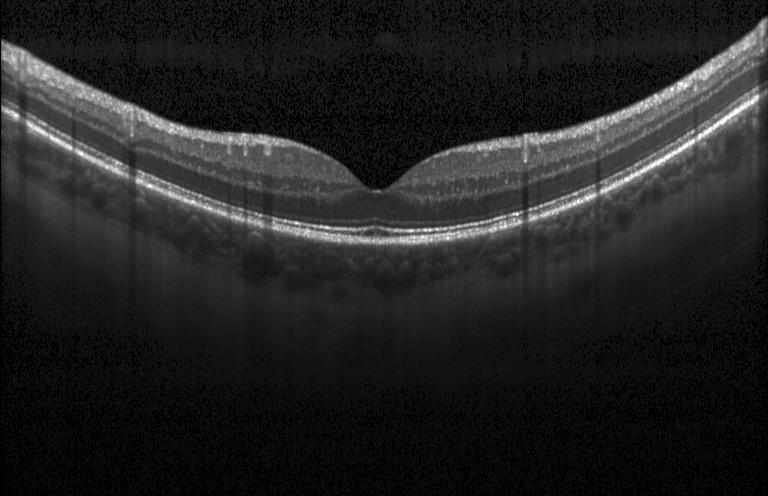
The scan shows no choroidal neovascularization, no diabetic macular edema, and no drusen.